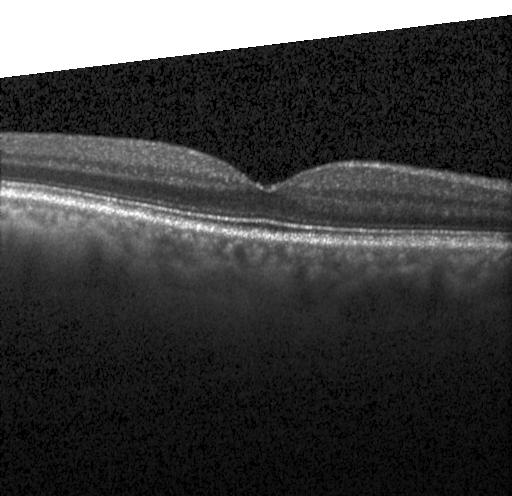

The scan shows no evidence of CNV, DME, or drusen.